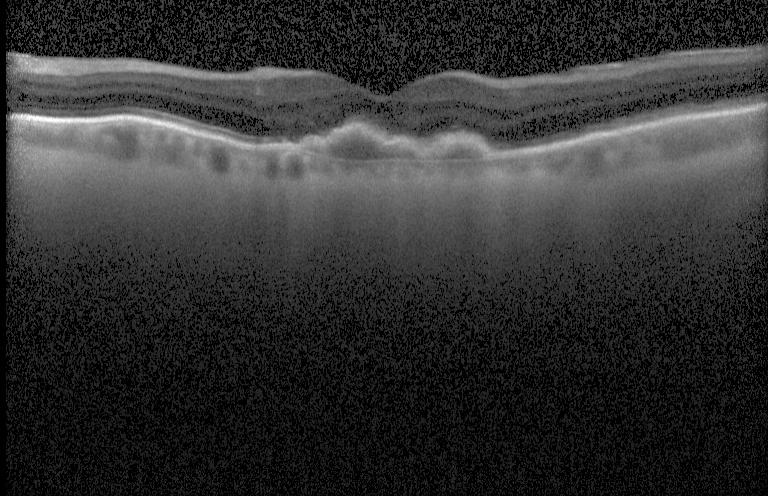 Diagnosis: a choroidal neovascular membrane.